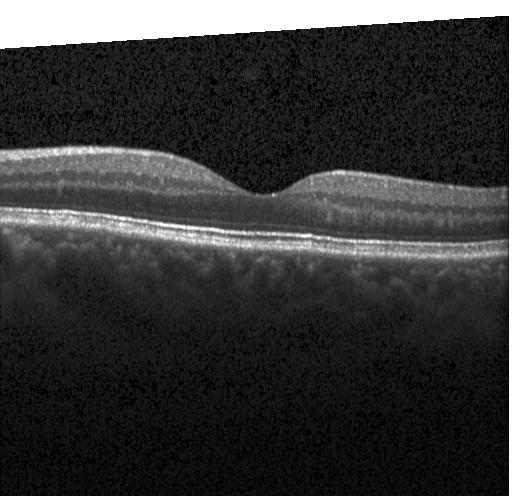
Impression: no choroidal neovascularization, no diabetic macular edema, and no drusen.